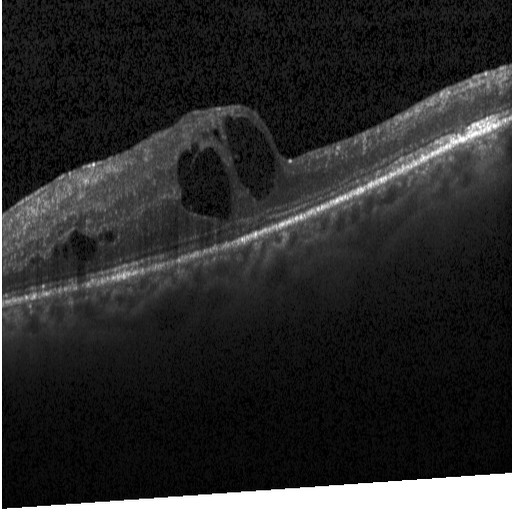 OCT line scan.
Finding: diabetic macular edema.